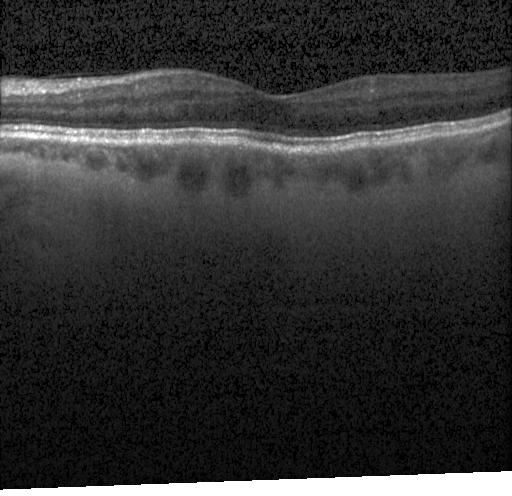
Macular OCT demonstrating neither CNV, DME, nor drusen.